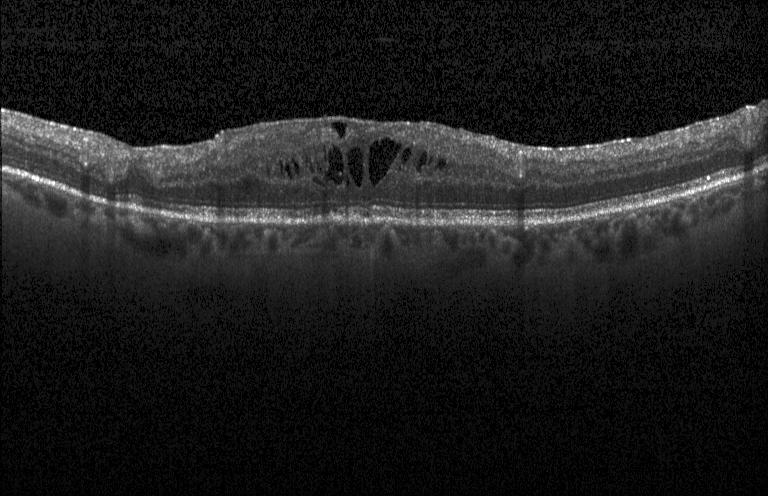

Heidelberg Spectralis. Retinal OCT B-scan. Spectral-domain optical coherence tomography. This B-scan demonstrates DME.